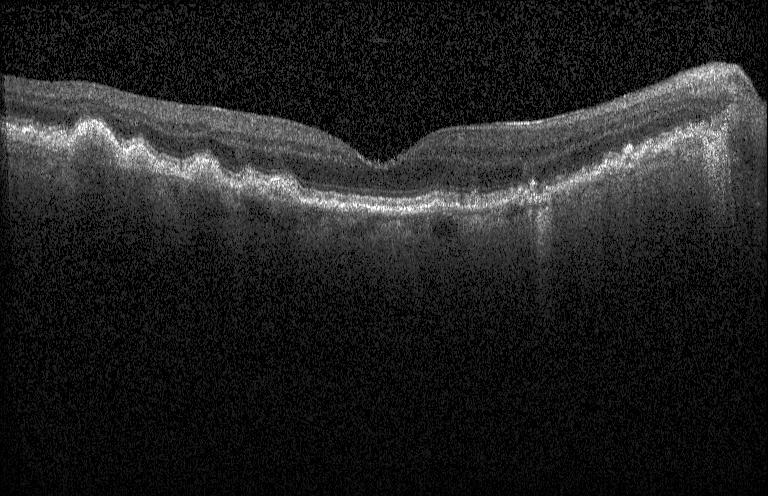 Macular scan; spectral-domain OCT; instrument: Heidelberg Spectralis; retinal OCT cross-section
Impression: sub-RPE drusenoid deposits.